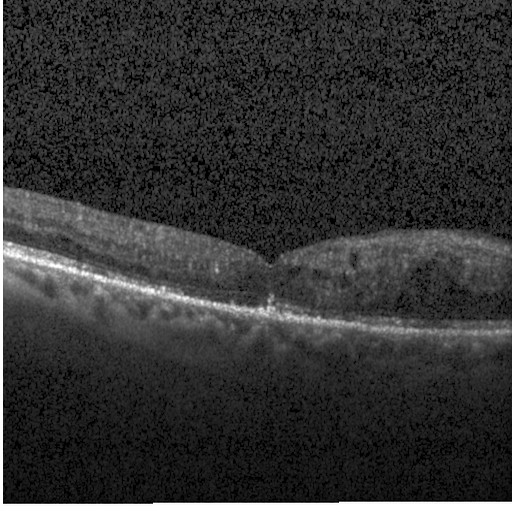 Retinal OCT cross-section. Impression: diabetic macular edema.